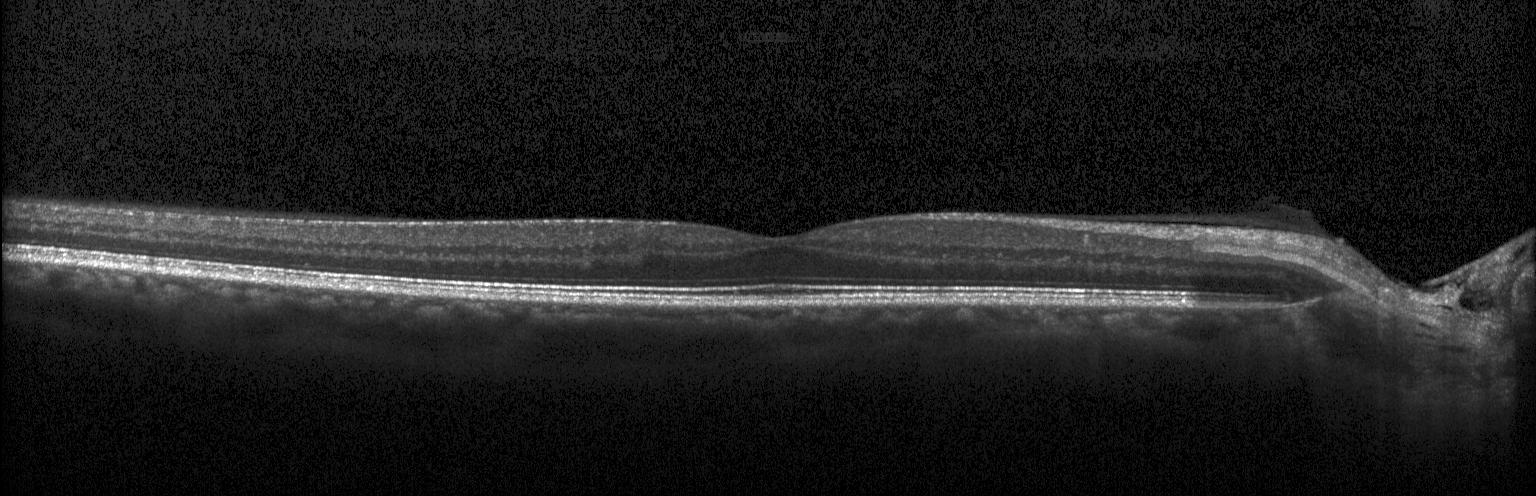
OCT B-scan. Macular OCT: neither CNV, DME, nor drusen.